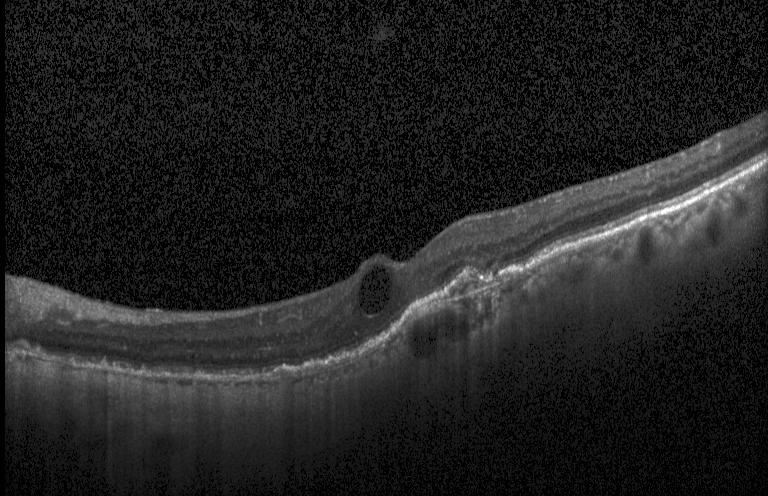
Acquired on a Heidelberg Spectralis, centered on the fovea, optical coherence tomography scan.
Impression: choroidal neovascularization.